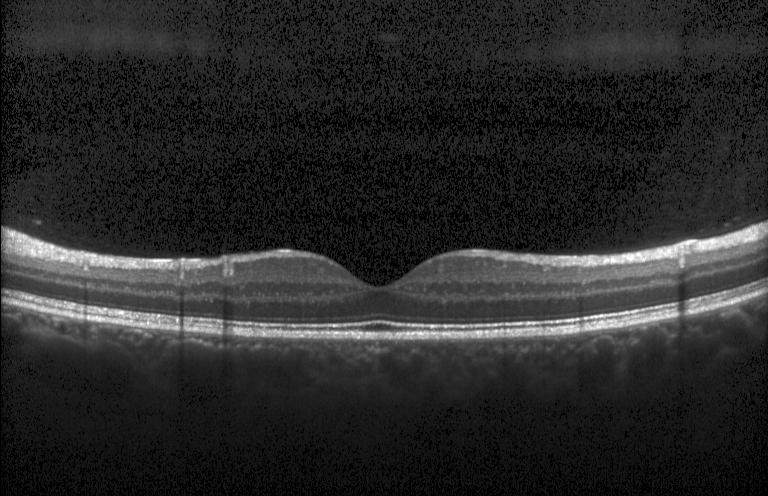 Retinal OCT cross-section
Diagnosis: no evidence of CNV, DME, or drusen.